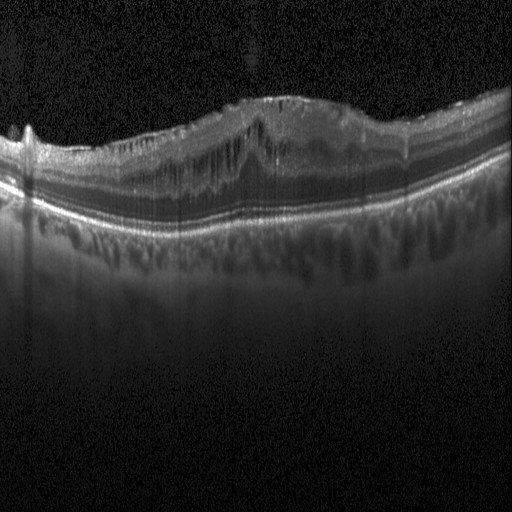

Centered on the fovea. Acquired on a Heidelberg Spectralis. Retinal OCT B-scan — Impression: diabetic macular edema (DME).